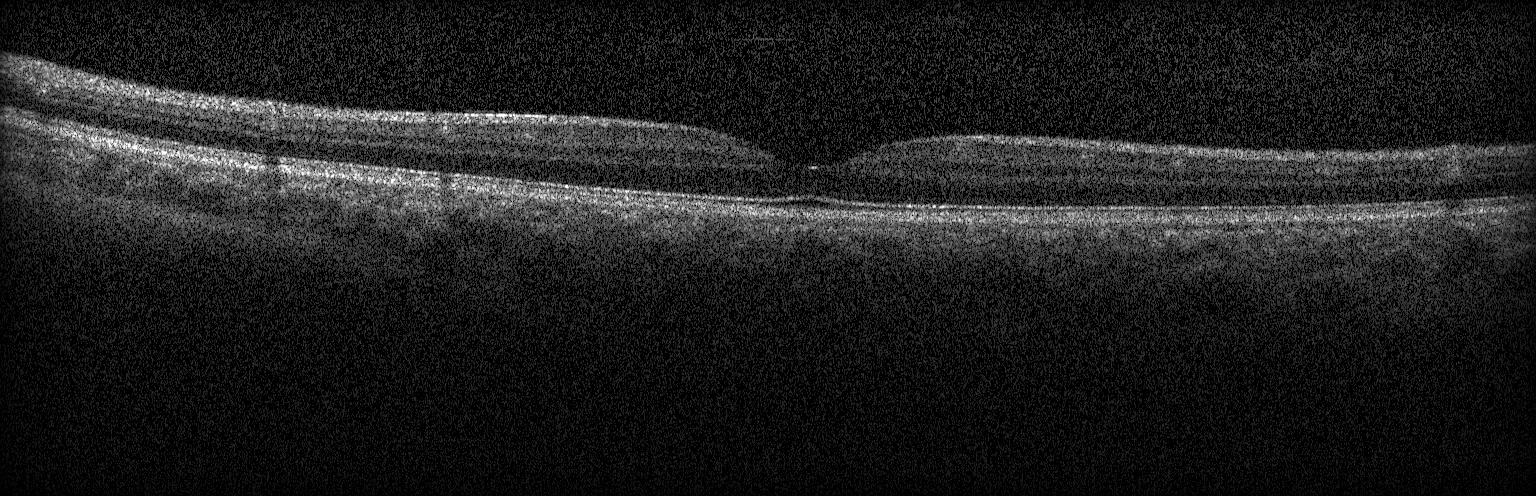 Spectral-domain OCT B-scan: no choroidal neovascularization, no diabetic macular edema, and no drusen.